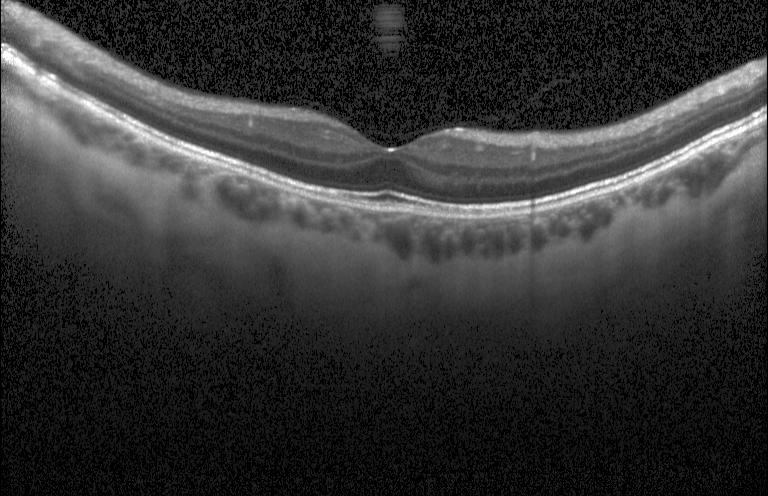

Diagnosis: neither CNV, DME, nor drusen.